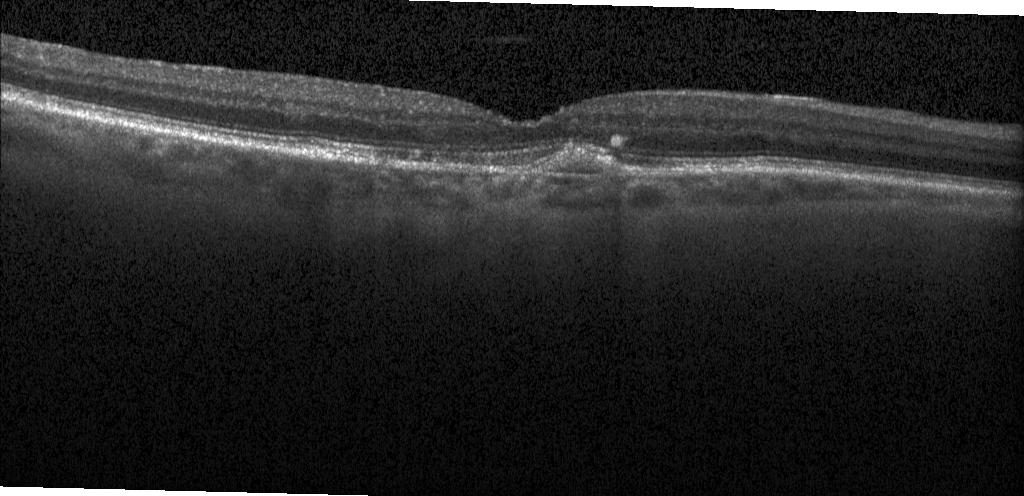 SD-OCT · optical coherence tomography B-scan.
Macular OCT: a choroidal neovascular membrane.